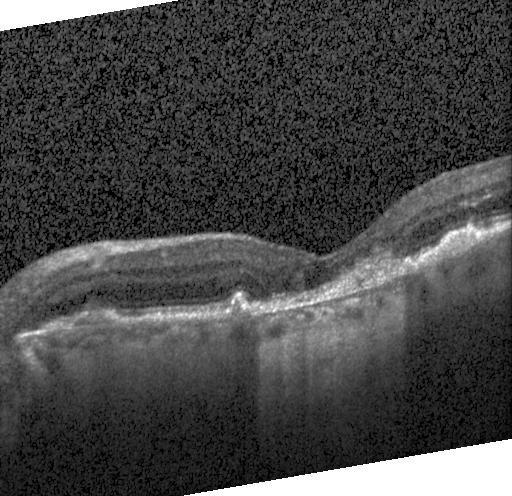
Heidelberg Spectralis OCT system. Optical coherence tomography scan
Assessment: a choroidal neovascular membrane.